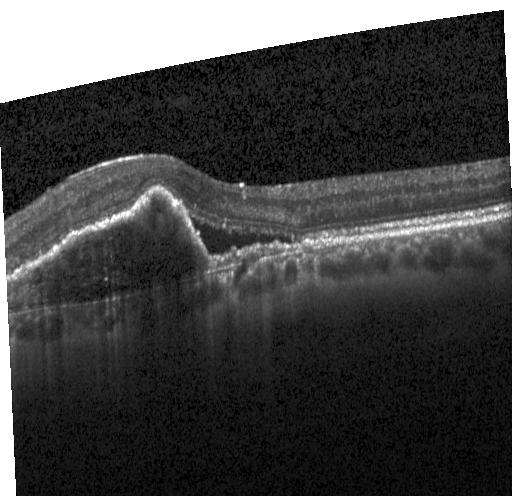

Acquired on a Heidelberg Spectralis; SD-OCT; fovea-centered; optical coherence tomography B-scan. OCT finding: a choroidal neovascular membrane.